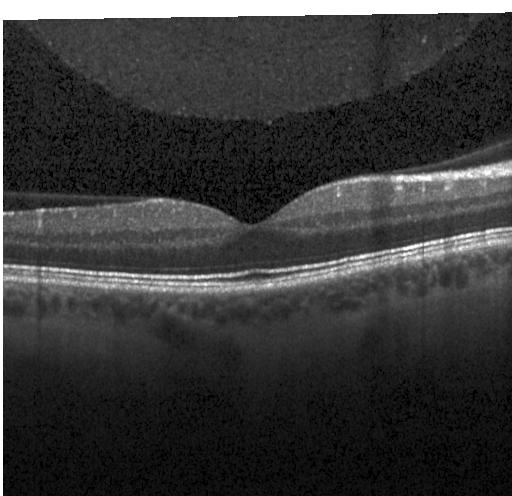

Optical coherence tomography scan.
Macular OCT: no evidence of choroidal neovascularization, diabetic macular edema, or drusen.